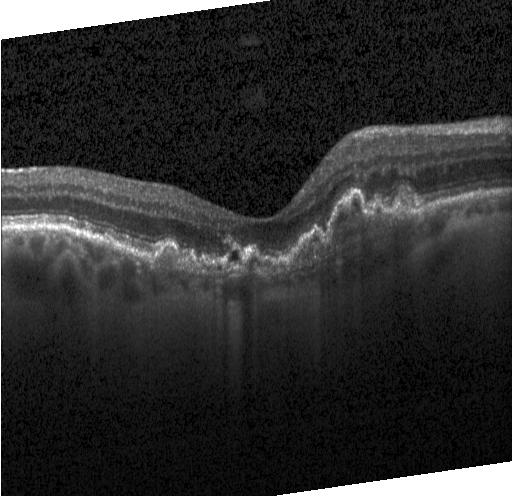 Heidelberg Spectralis OCT system; fovea-centered; OCT B-scan
Choroidal neovascularization.